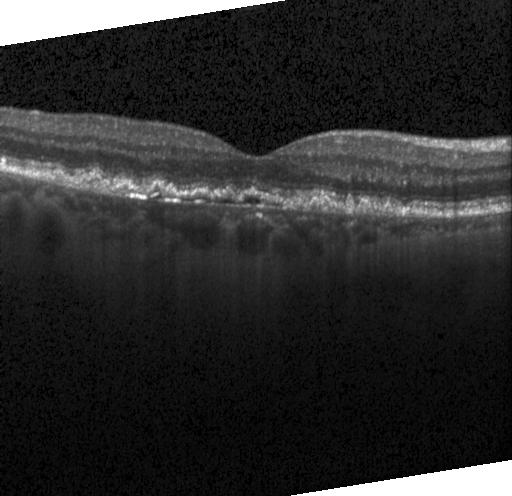
Diagnosis: CNV.